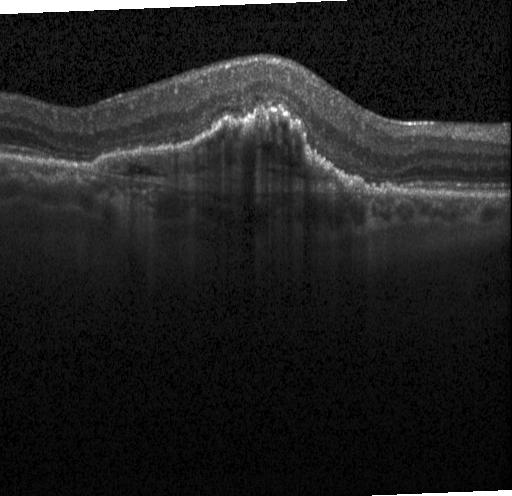

Fovea-centered; optical coherence tomography scan; Heidelberg Spectralis; SD-OCT — Macular OCT: choroidal neovascularization.